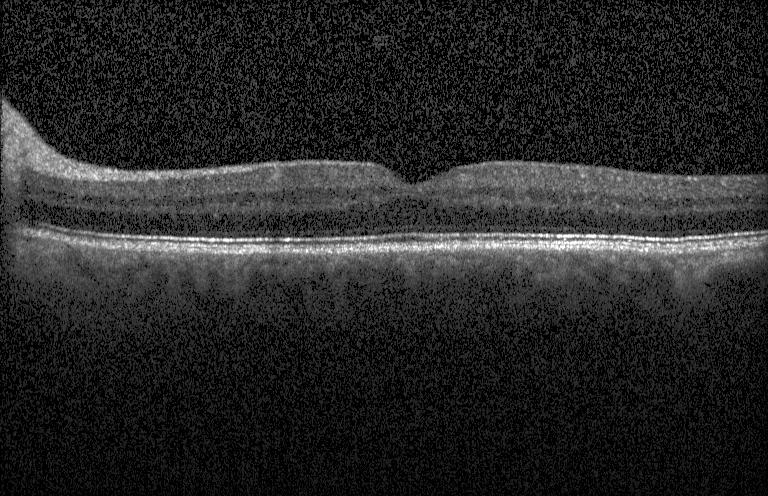

Optical coherence tomography B-scan. Diagnosis: no CNV, DME, or drusen.